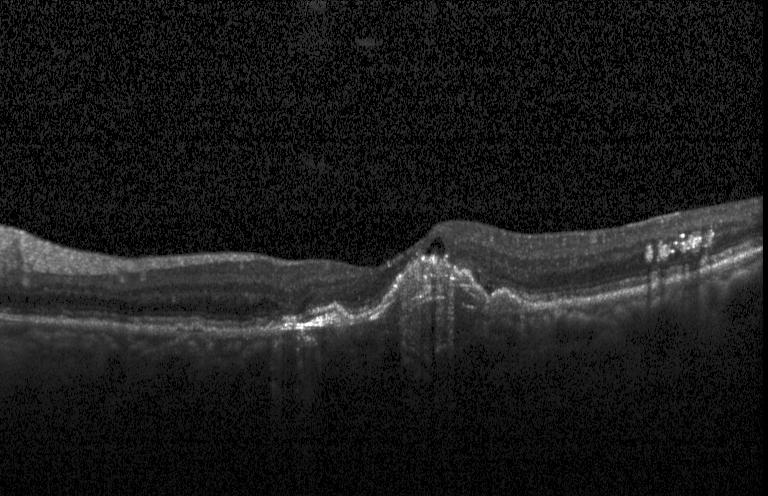
Spectral-domain optical coherence tomography; optical coherence tomography B-scan. Finding: CNV.